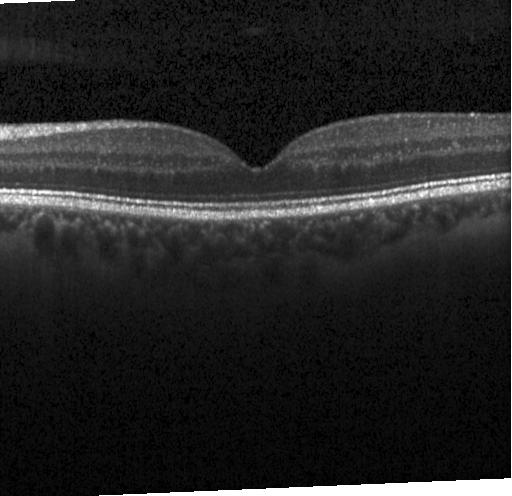

Heidelberg Spectralis; OCT line scan; spectral-domain OCT. Impression: no choroidal neovascularization, diabetic macular edema, or drusen.